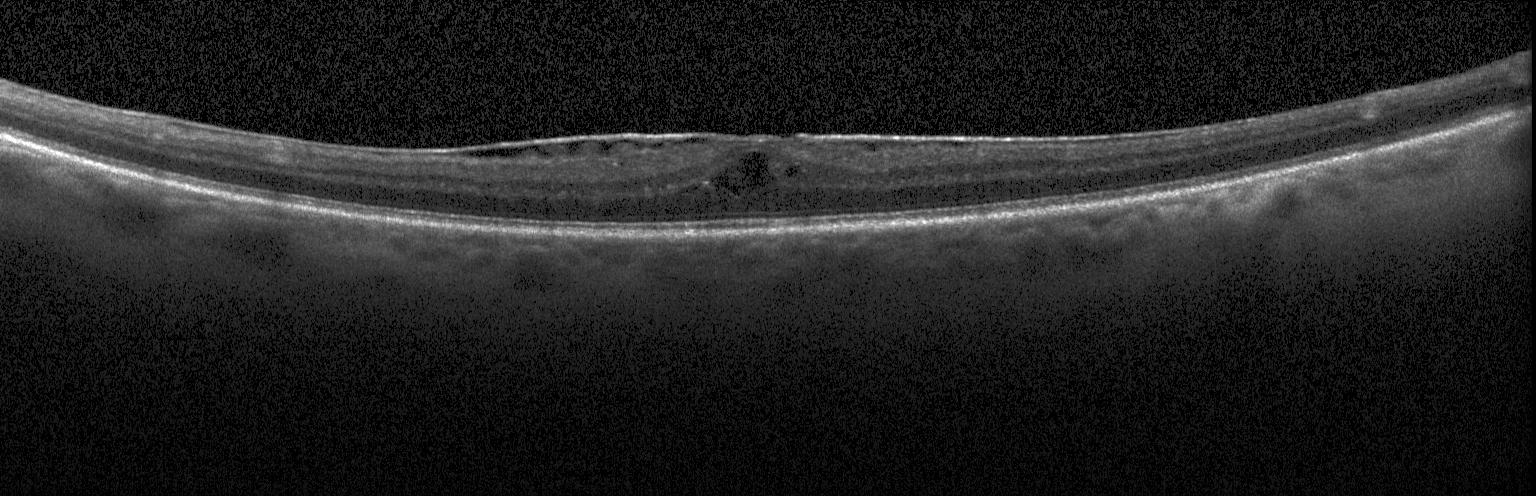
Spectral-domain optical coherence tomography, OCT line scan, through the macula
Diabetic macular edema (DME).